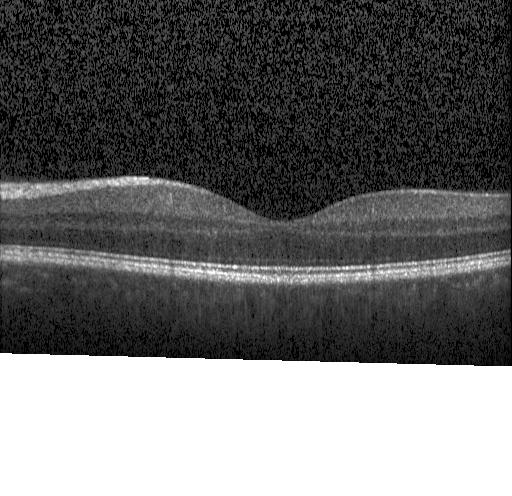

OCT finding: no evidence of CNV, DME, or drusen.